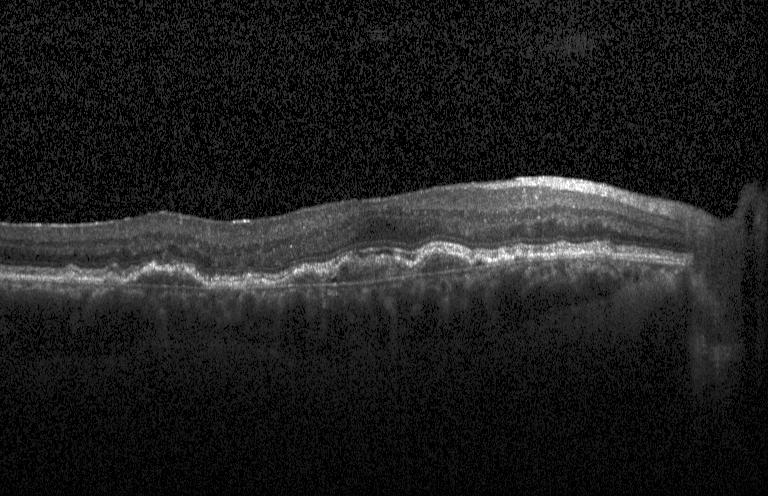
Diagnosis: a choroidal neovascular membrane.